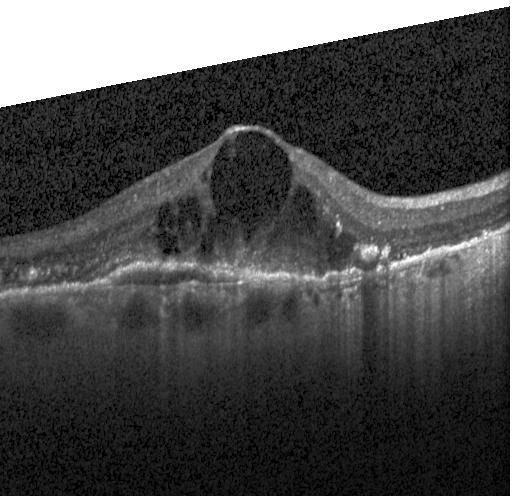 Finding: choroidal neovascularization (CNV).